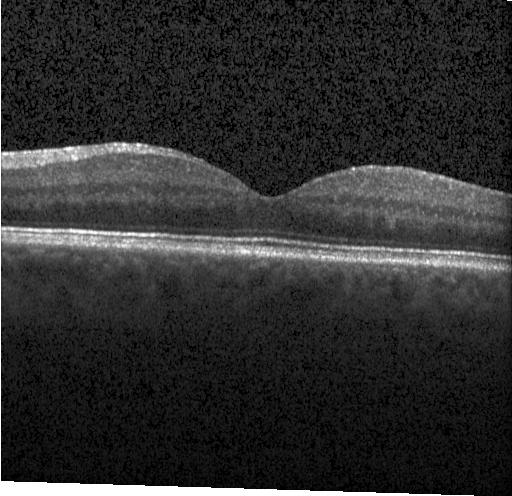 Spectral-domain OCT B-scan: neither choroidal neovascularization, diabetic macular edema, nor drusen.